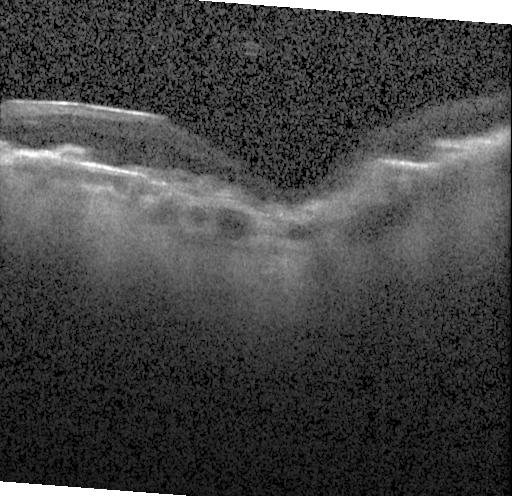
Instrument: Heidelberg Spectralis · horizontal scan through the fovea · spectral-domain OCT · optical coherence tomography scan — Choroidal neovascularization.